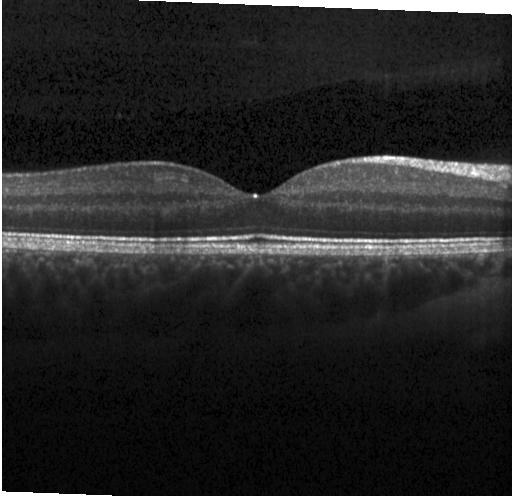 Optical coherence tomography B-scan · Heidelberg Spectralis OCT system · spectral-domain OCT · horizontal scan through the fovea.
Impression: no evidence of choroidal neovascularization, diabetic macular edema, or drusen.